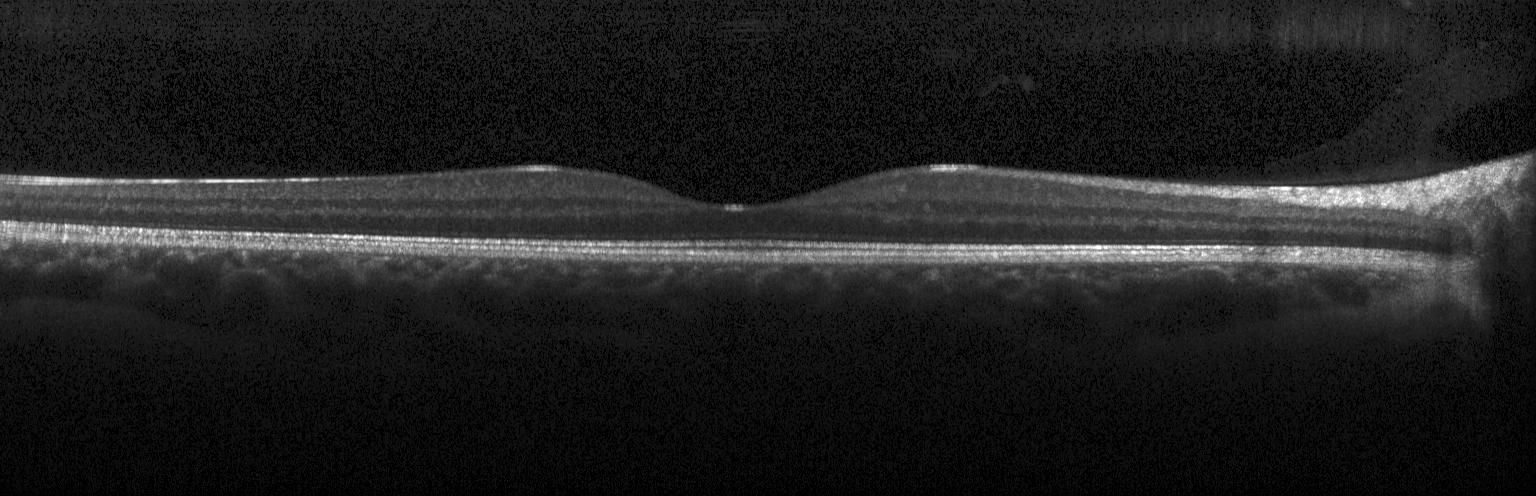 OCT line scan, SD-OCT. Diagnosis: neither CNV, DME, nor drusen.